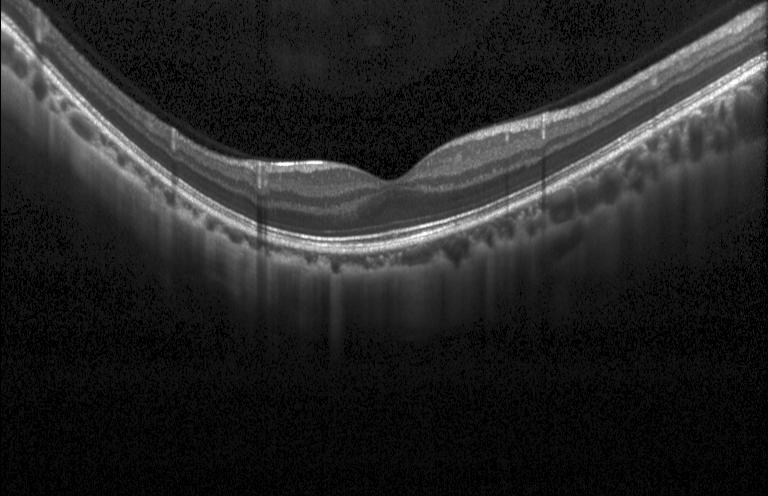
Macular OCT demonstrating no choroidal neovascularization, no diabetic macular edema, and no drusen.